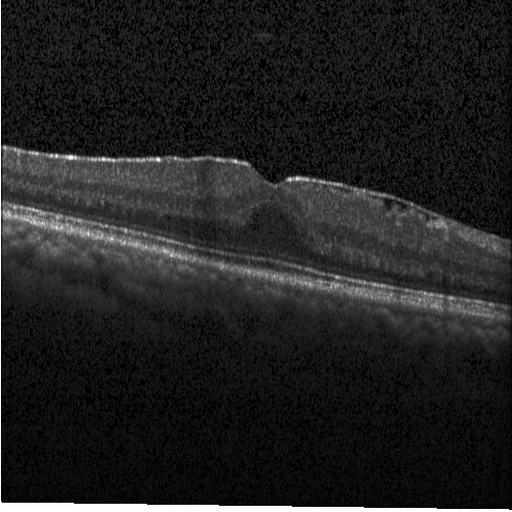 Dx: diabetic macular edema (DME).